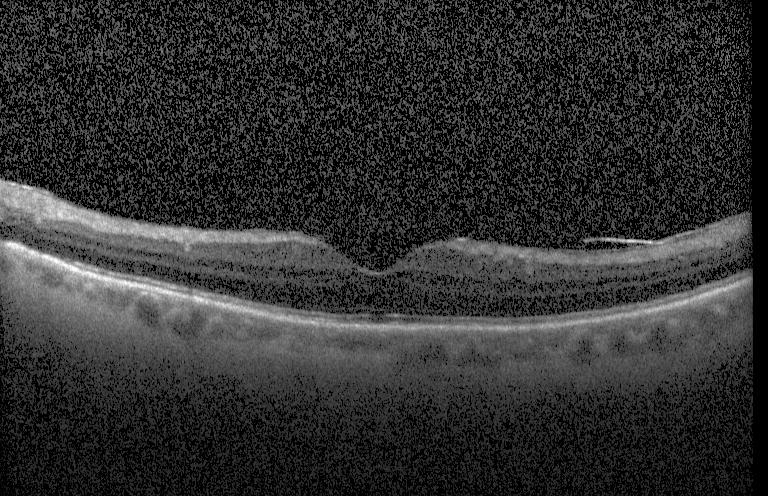 OCT B-scan. Macular OCT: no evidence of choroidal neovascularization, diabetic macular edema, or drusen.